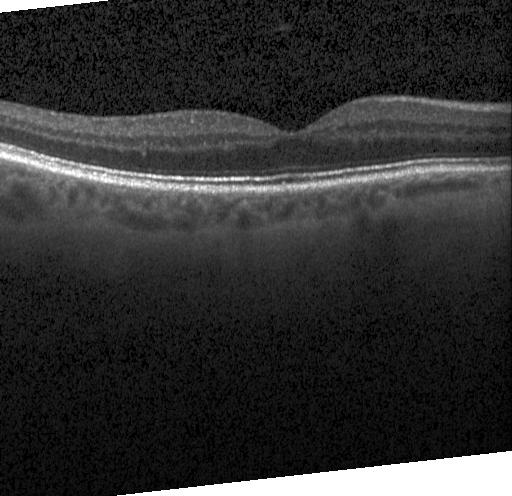
This B-scan demonstrates no evidence of choroidal neovascularization, diabetic macular edema, or drusen.